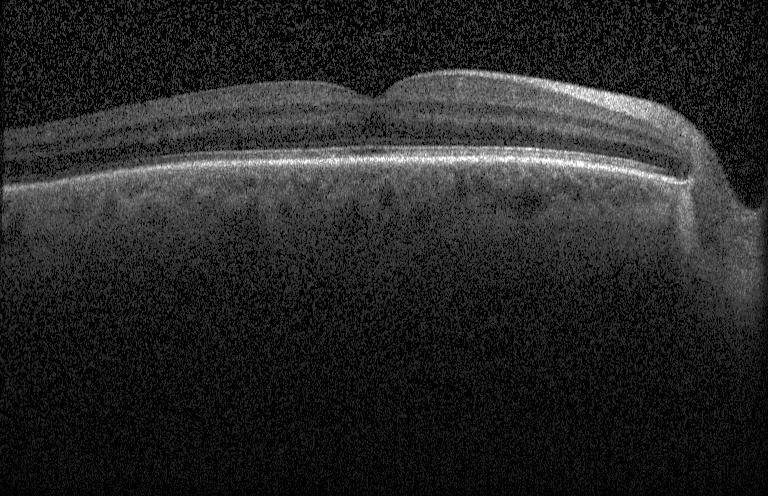 Assessment: no CNV, no DME, and no drusen.